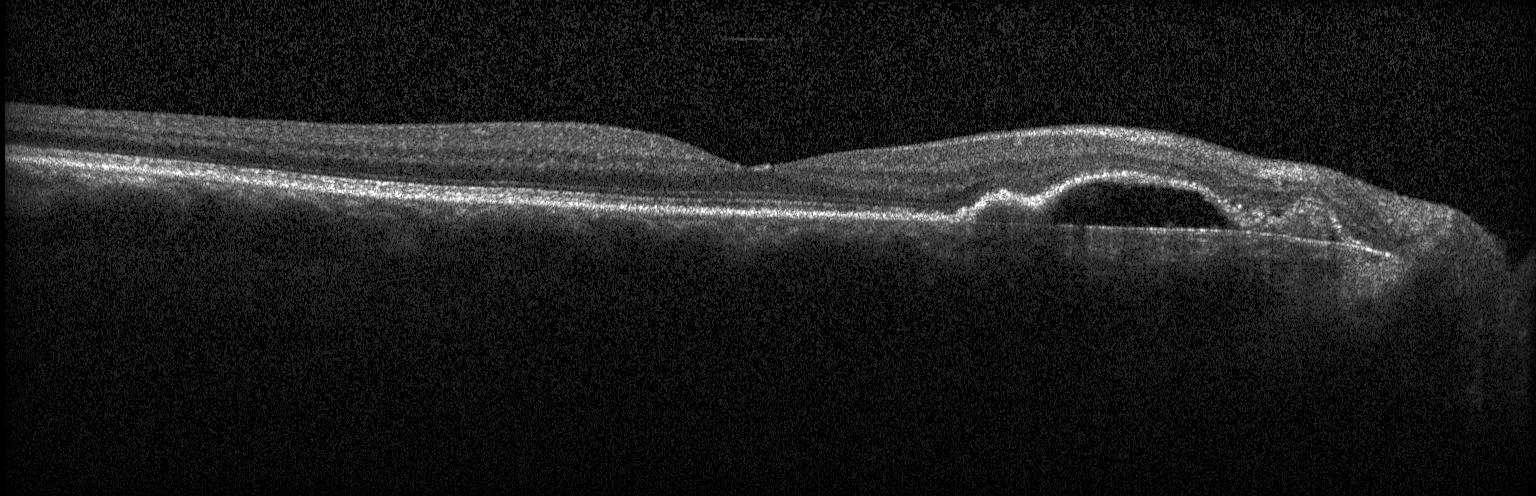
Finding: CNV.